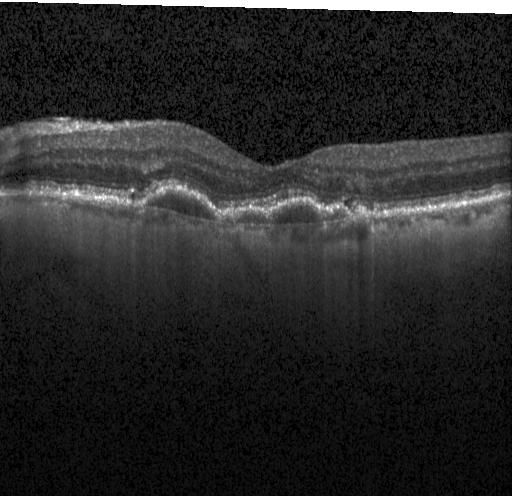
Fovea-centered; retinal OCT B-scan. Macular OCT: choroidal neovascularization (CNV).